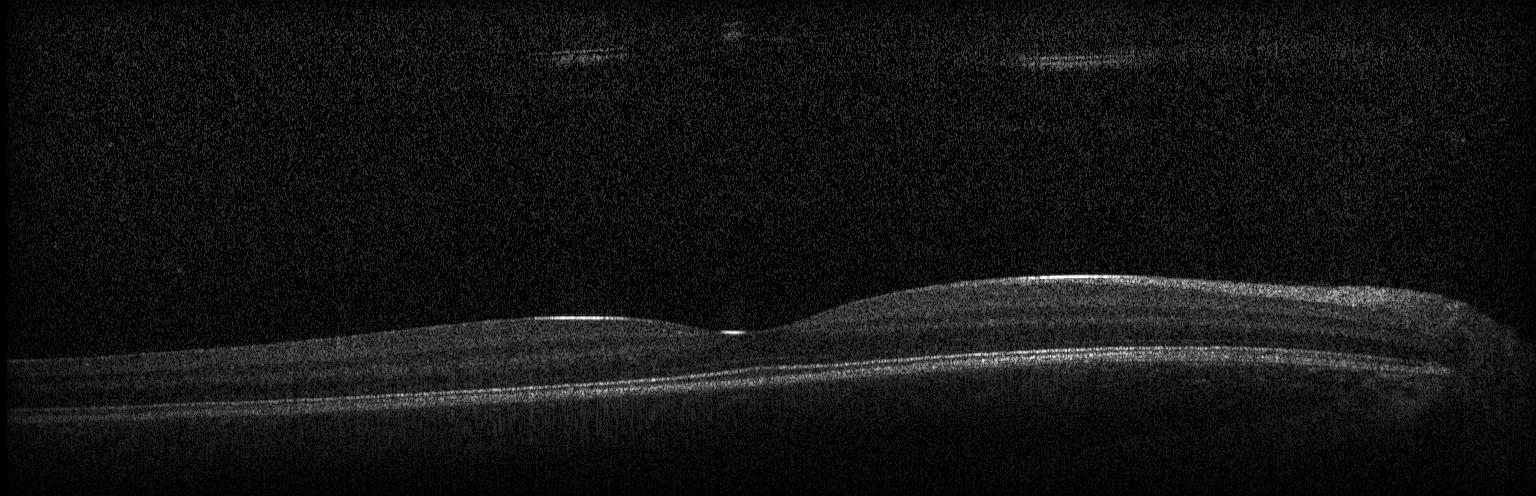
OCT B-scan
Finding: neither choroidal neovascularization, diabetic macular edema, nor drusen.